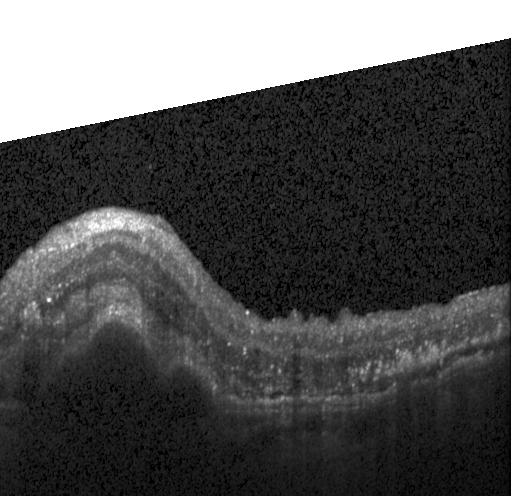

The scan shows choroidal neovascularization (CNV).